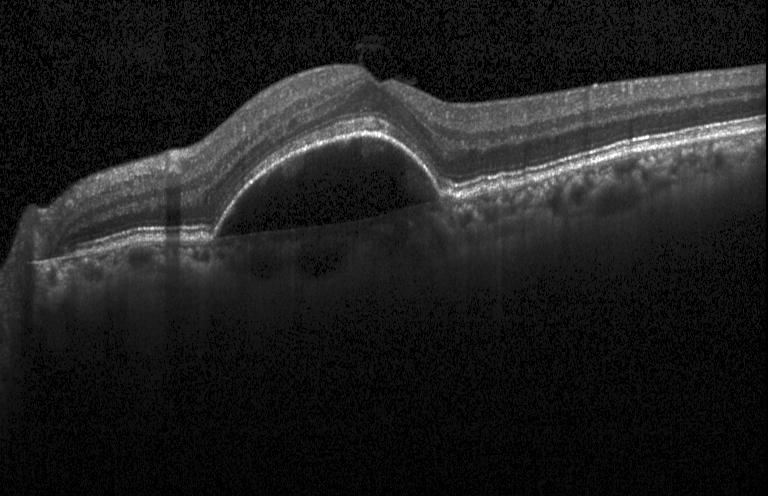 Horizontal scan through the fovea. Acquired on a Heidelberg Spectralis. Spectral-domain OCT. OCT line scan
Diagnosis: a choroidal neovascular membrane.